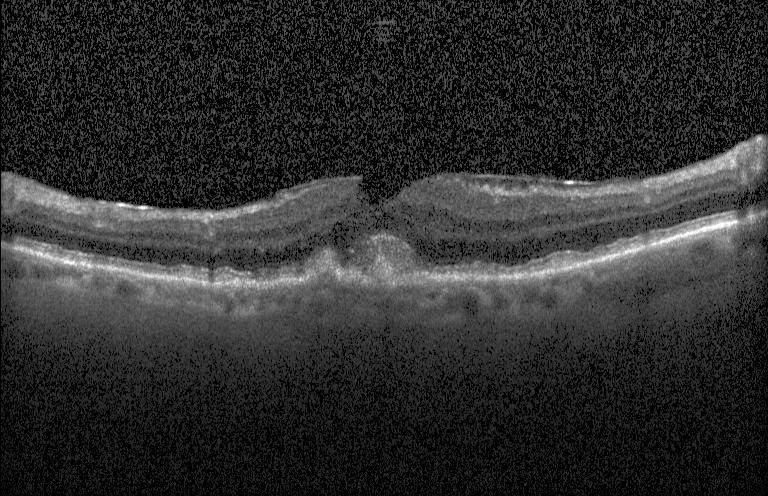 OCT finding: a choroidal neovascular membrane.